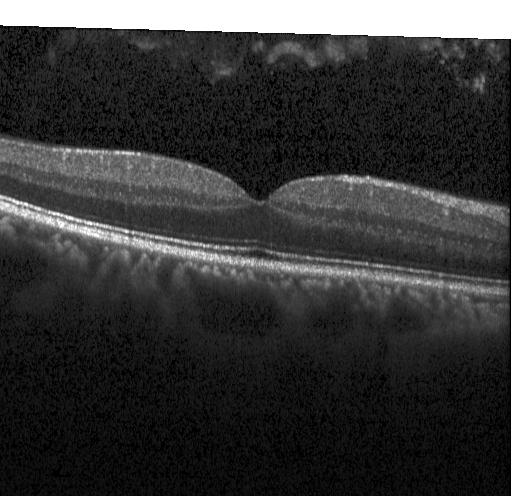 Retinal OCT B-scan
Macular OCT: neither CNV, DME, nor drusen.